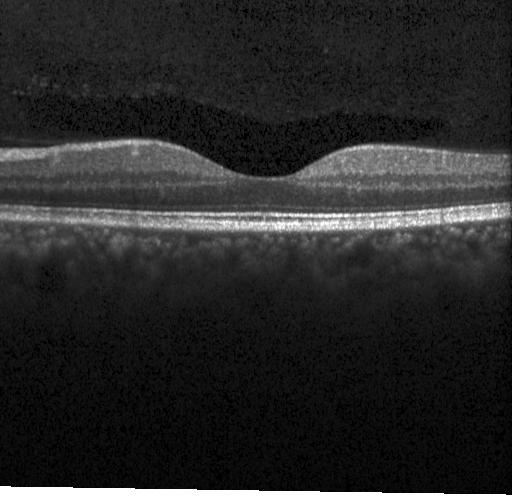

Heidelberg Spectralis OCT system · spectral-domain OCT · macular scan · retinal OCT cross-section
Neither CNV, DME, nor drusen.